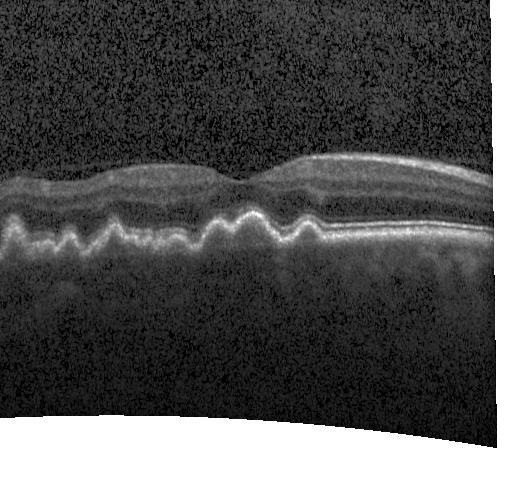
Retinal OCT cross-section; through the macula; acquired on a Heidelberg Spectralis. Finding: sub-RPE drusenoid deposits.